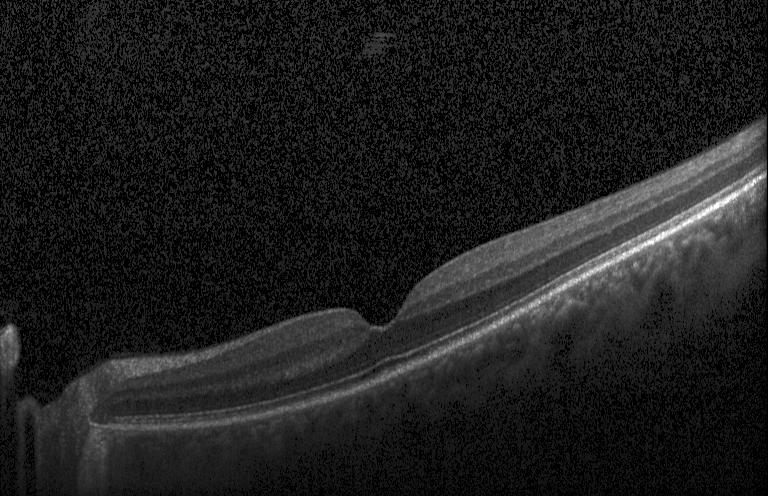

Acquired on a Heidelberg Spectralis, optical coherence tomography B-scan, spectral-domain OCT, horizontal scan through the fovea. Neither choroidal neovascularization, diabetic macular edema, nor drusen.